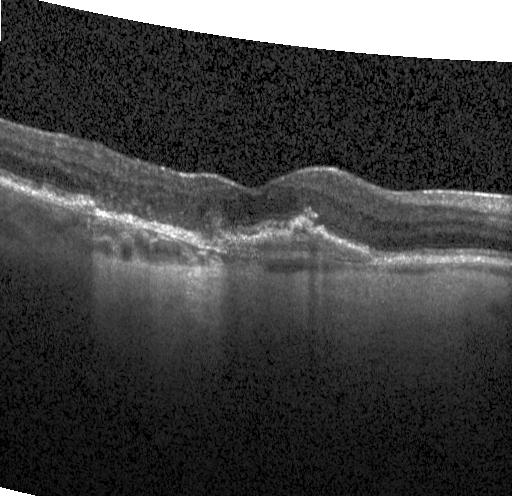 Instrument: Heidelberg Spectralis, optical coherence tomography B-scan
Diagnosis: choroidal neovascularization (CNV).